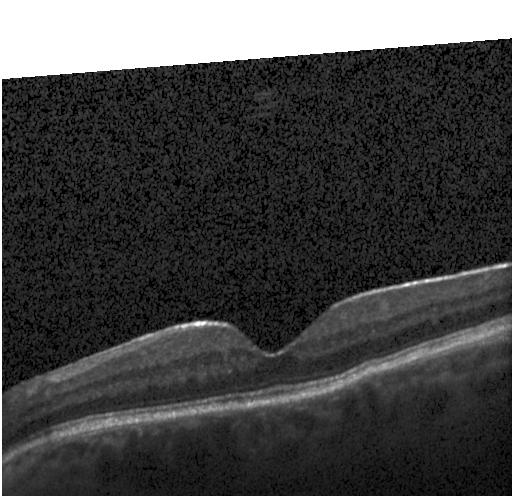

Impression: no CNV, no DME, and no drusen.